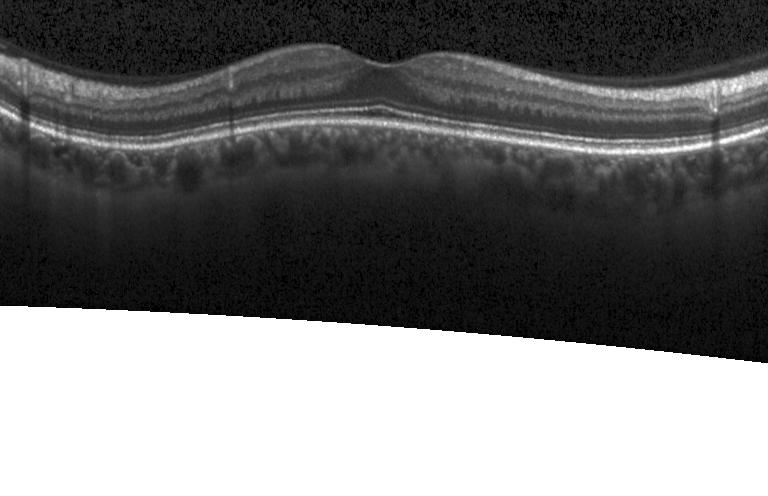

Retinal OCT cross-section showing no evidence of choroidal neovascularization, diabetic macular edema, or drusen.